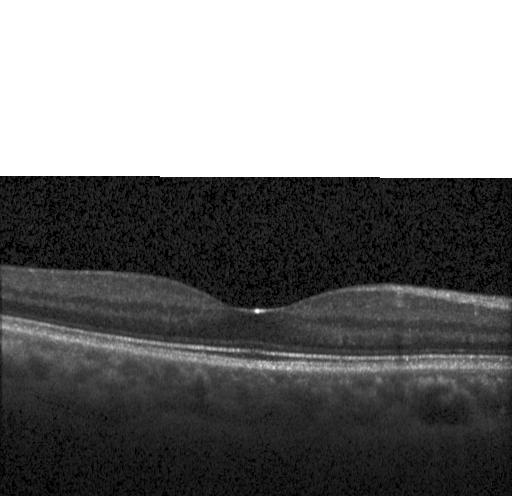

Assessment: neither choroidal neovascularization, diabetic macular edema, nor drusen.